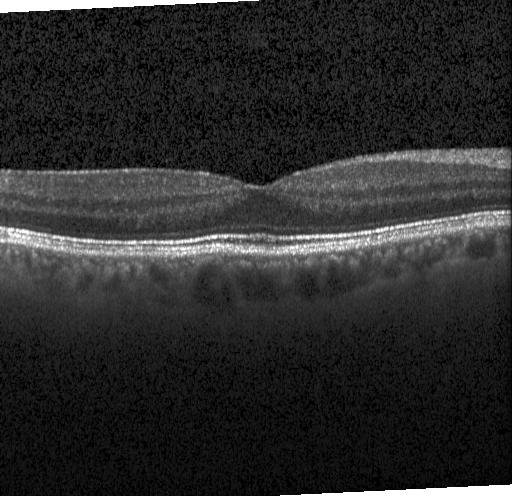

Macular OCT demonstrating no CNV, no DME, and no drusen.